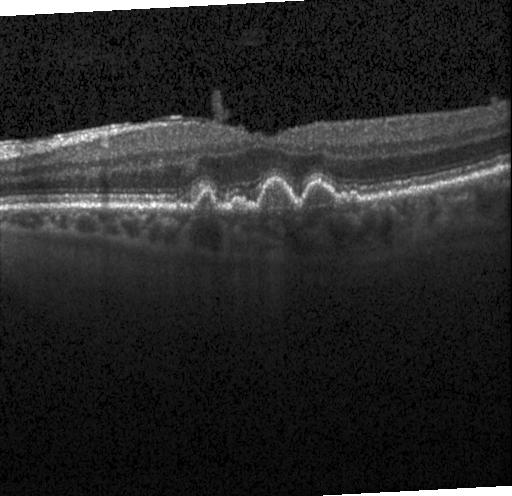

Diagnosis: multiple drusen.